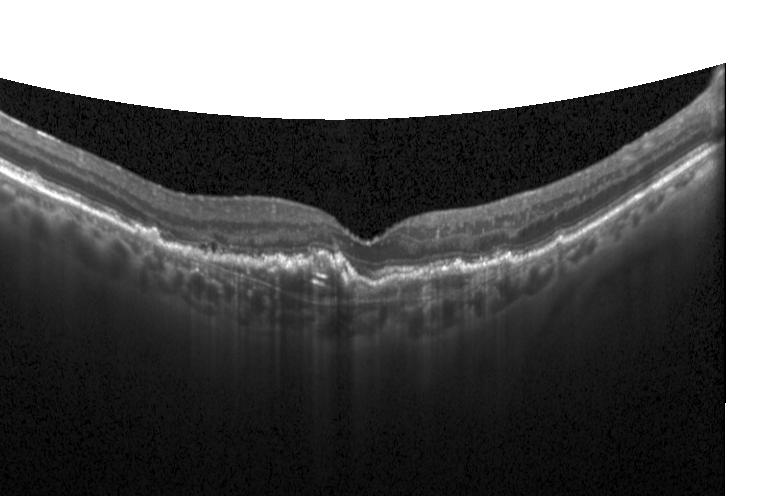 Heidelberg Spectralis OCT system, optical coherence tomography B-scan, spectral-domain OCT, through the macula
The scan shows a choroidal neovascular membrane.